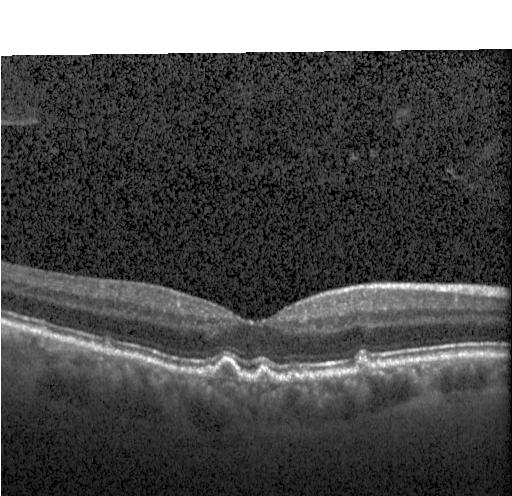 Retinal OCT B-scan, Heidelberg Spectralis OCT system. Dx: drusen.